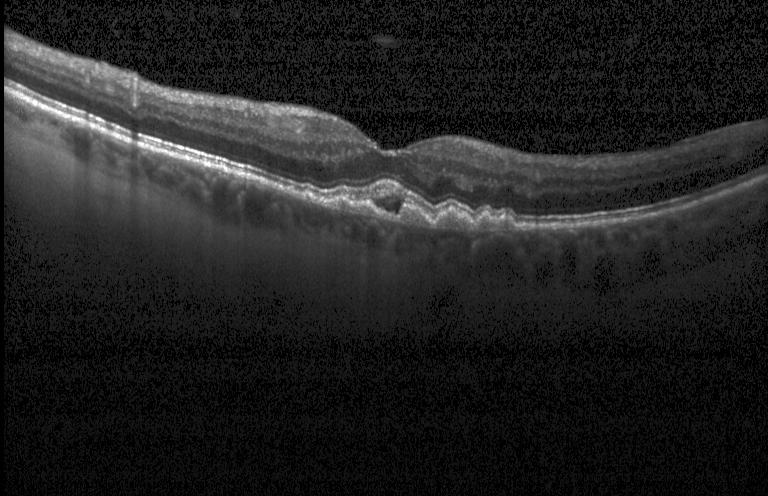

OCT B-scan; instrument: Heidelberg Spectralis; through the macula. Impression: multiple drusen.